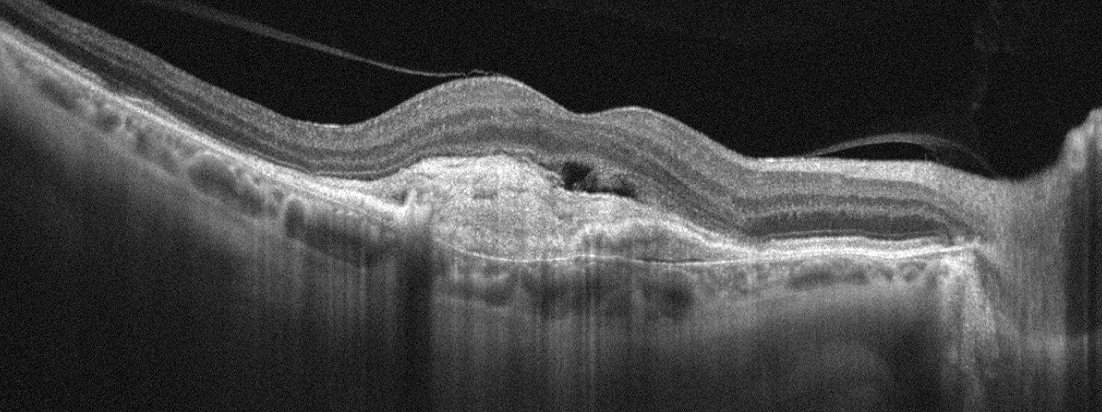

OCT B-scan
The scan shows age-related macular degeneration.